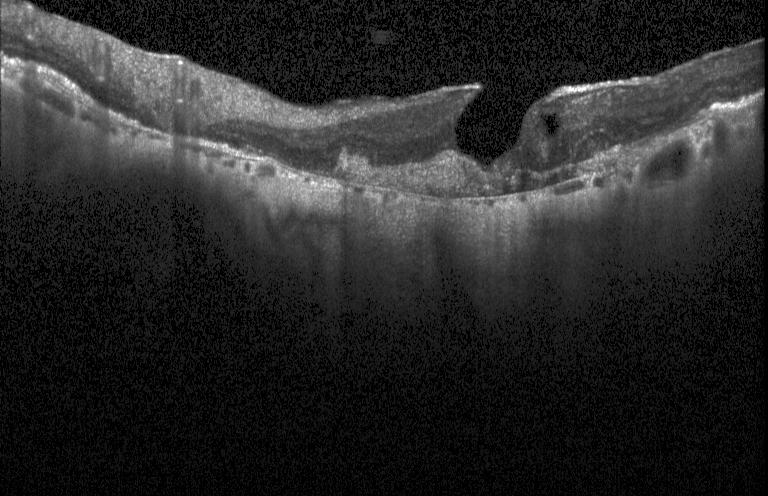
Optical coherence tomography scan. Fovea-centered. Instrument: Heidelberg Spectralis
Dx: a choroidal neovascular membrane.